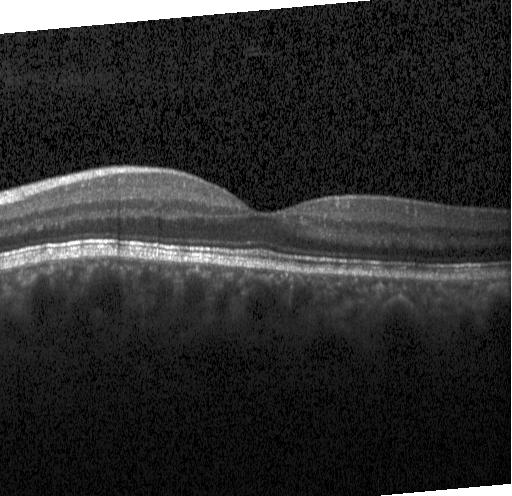

The scan shows neither choroidal neovascularization, diabetic macular edema, nor drusen.